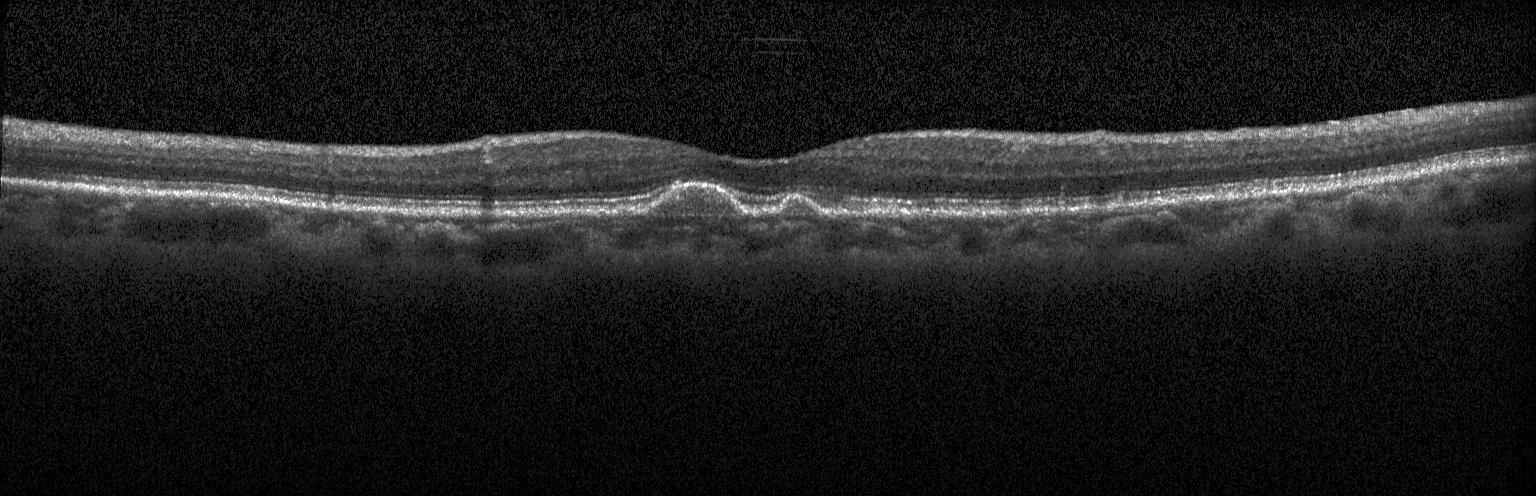 Fovea-centered. Instrument: Heidelberg Spectralis. Retinal OCT B-scan. Spectral-domain OCT — Diagnosis: sub-RPE drusenoid deposits.